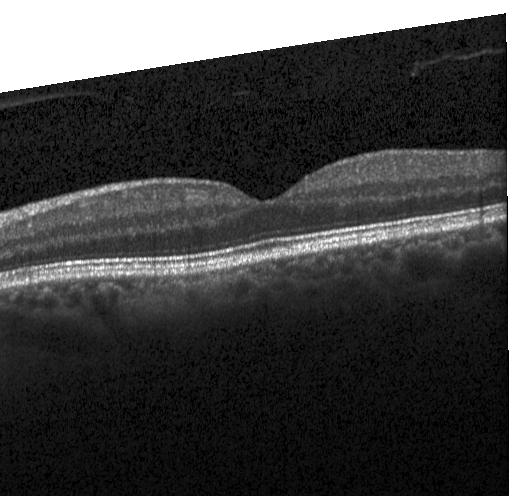 Diagnosis: no evidence of choroidal neovascularization, diabetic macular edema, or drusen.